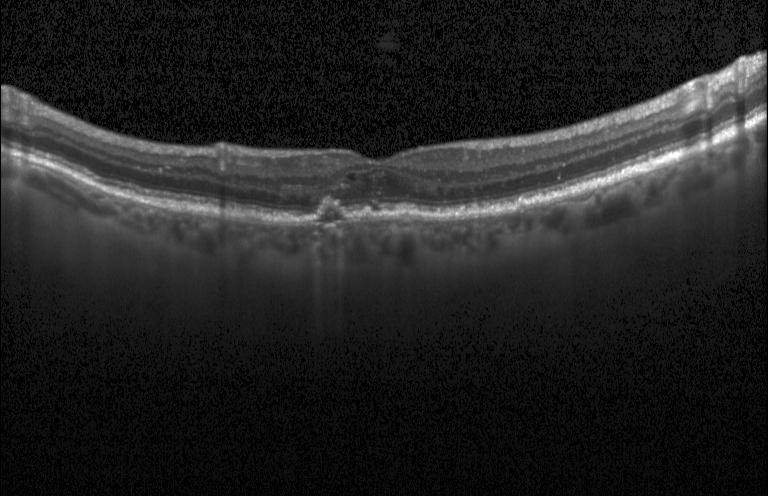
Acquired on a Heidelberg Spectralis · horizontal scan through the fovea · OCT B-scan · SD-OCT
OCT finding: a choroidal neovascular membrane.